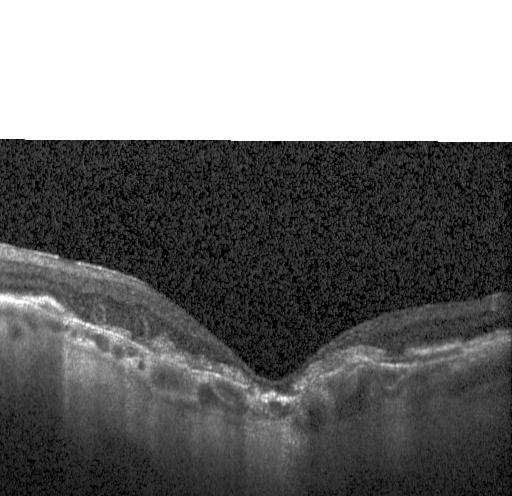

Optical coherence tomography B-scan, spectral-domain OCT. This B-scan demonstrates a choroidal neovascular membrane.